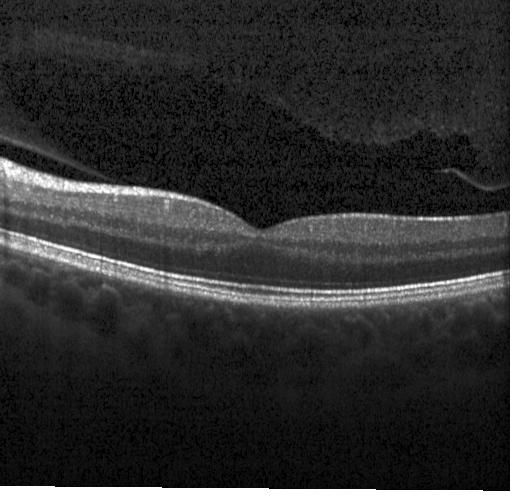
Spectral-domain OCT B-scan: no CNV, no DME, and no drusen.